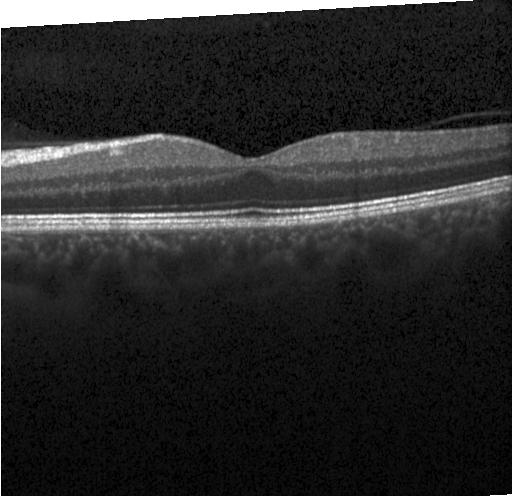
Spectral-domain OCT B-scan: no CNV, DME, or drusen.